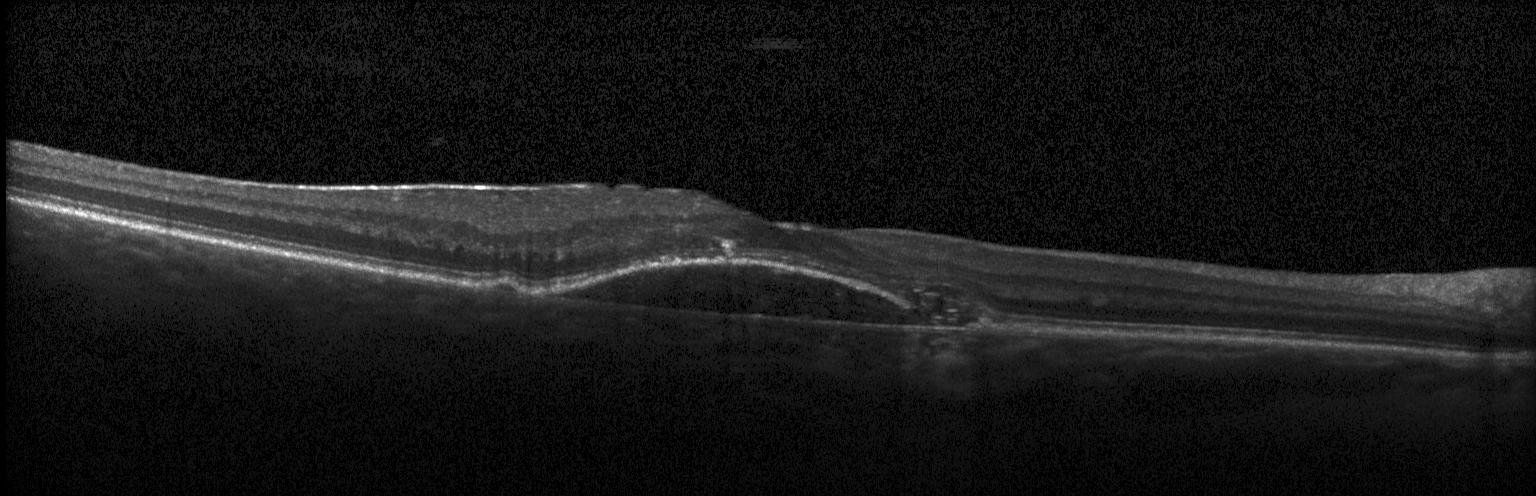
Heidelberg Spectralis OCT system · OCT line scan · spectral-domain OCT.
Diagnosis: a choroidal neovascular membrane.